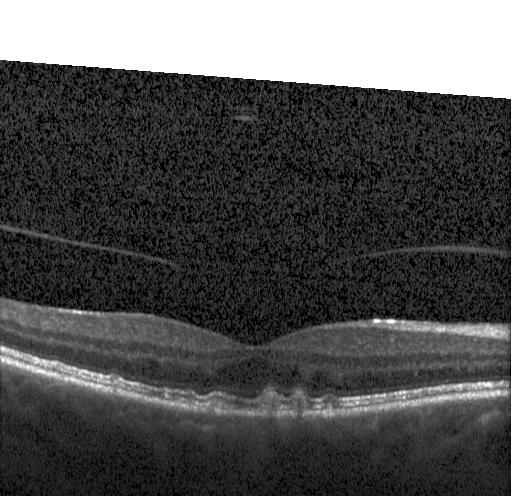

Retinal OCT cross-section
OCT finding: multiple drusen.